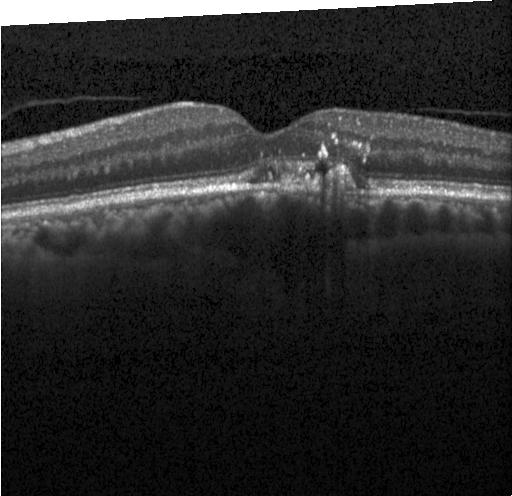

OCT line scan; fovea-centered; spectral-domain optical coherence tomography; Heidelberg Spectralis OCT system. The scan shows choroidal neovascularization.